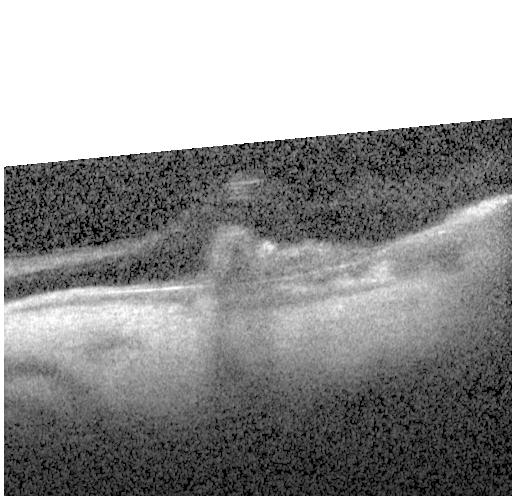

The scan shows a choroidal neovascular membrane.